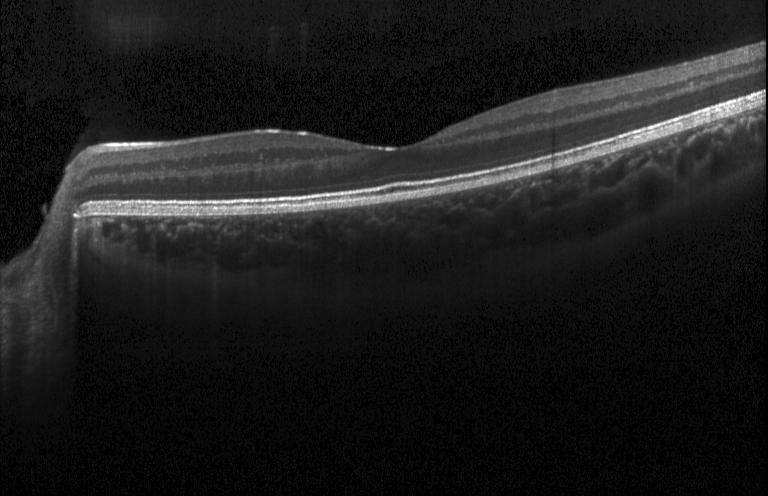

Optical coherence tomography scan; spectral-domain OCT.
No choroidal neovascularization, no diabetic macular edema, and no drusen.